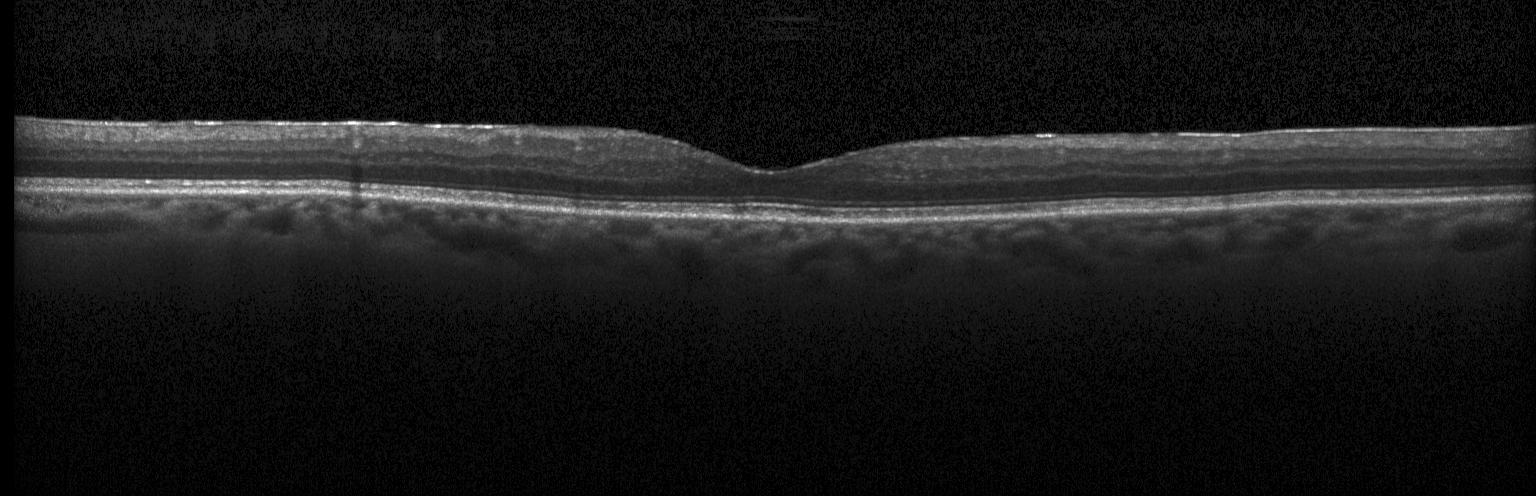
Heidelberg Spectralis, OCT B-scan. Macular OCT: no choroidal neovascularization, diabetic macular edema, or drusen.